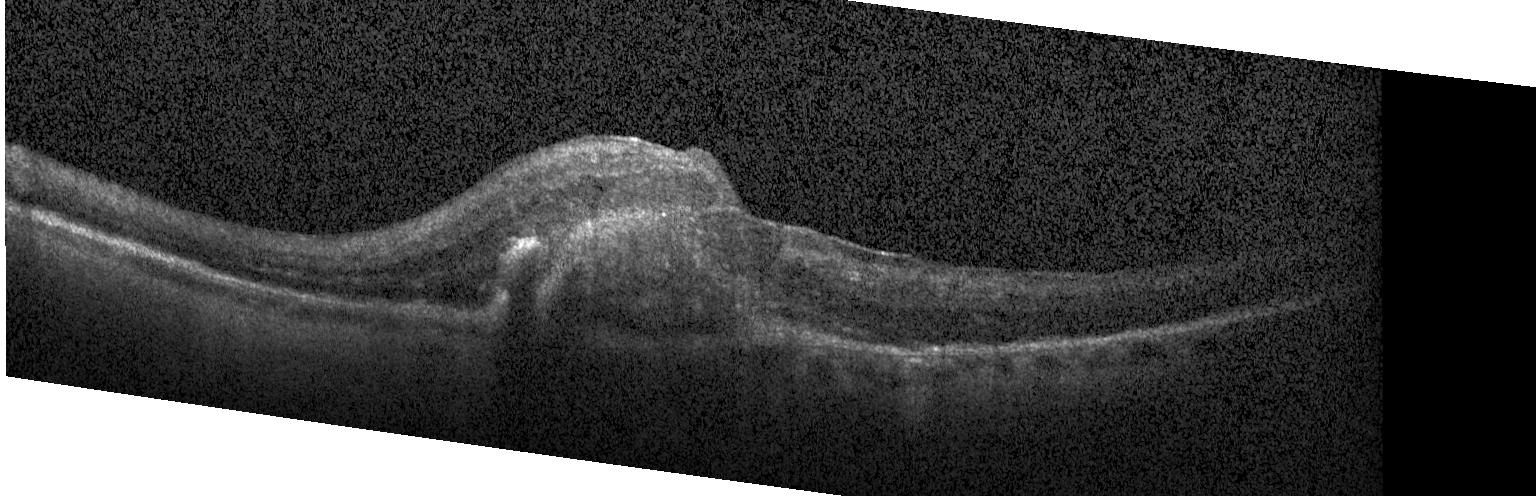 OCT scan showing CNV.